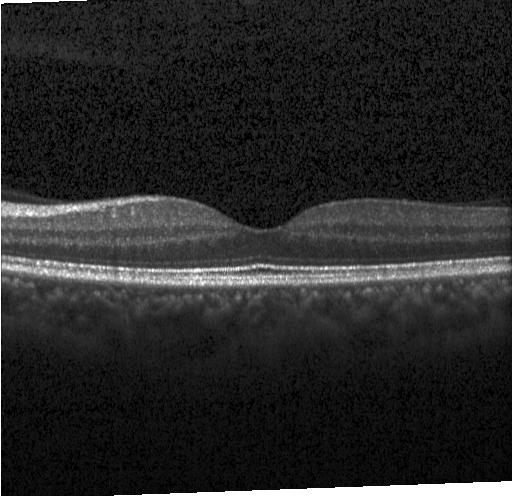

Retinal OCT cross-section. Macular OCT: no choroidal neovascularization, diabetic macular edema, or drusen.